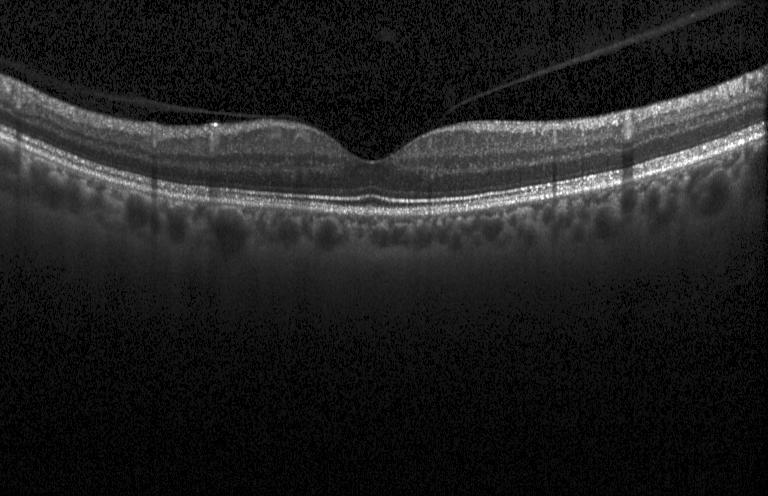 OCT B-scan
The scan shows no choroidal neovascularization, diabetic macular edema, or drusen.